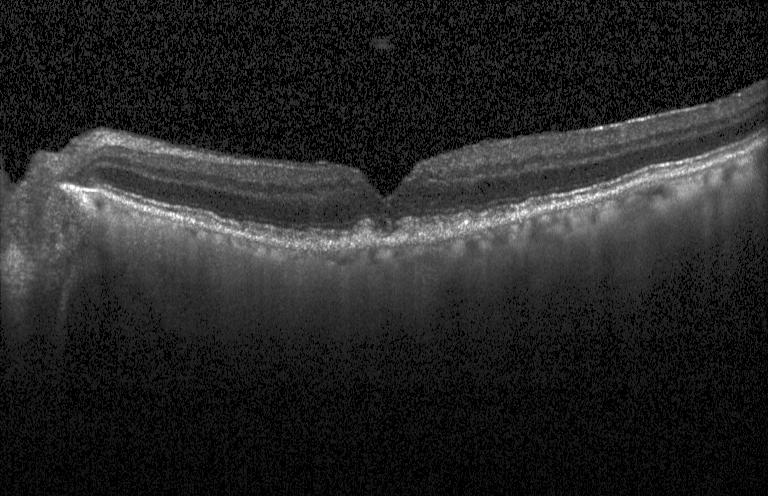
Assessment: drusen.